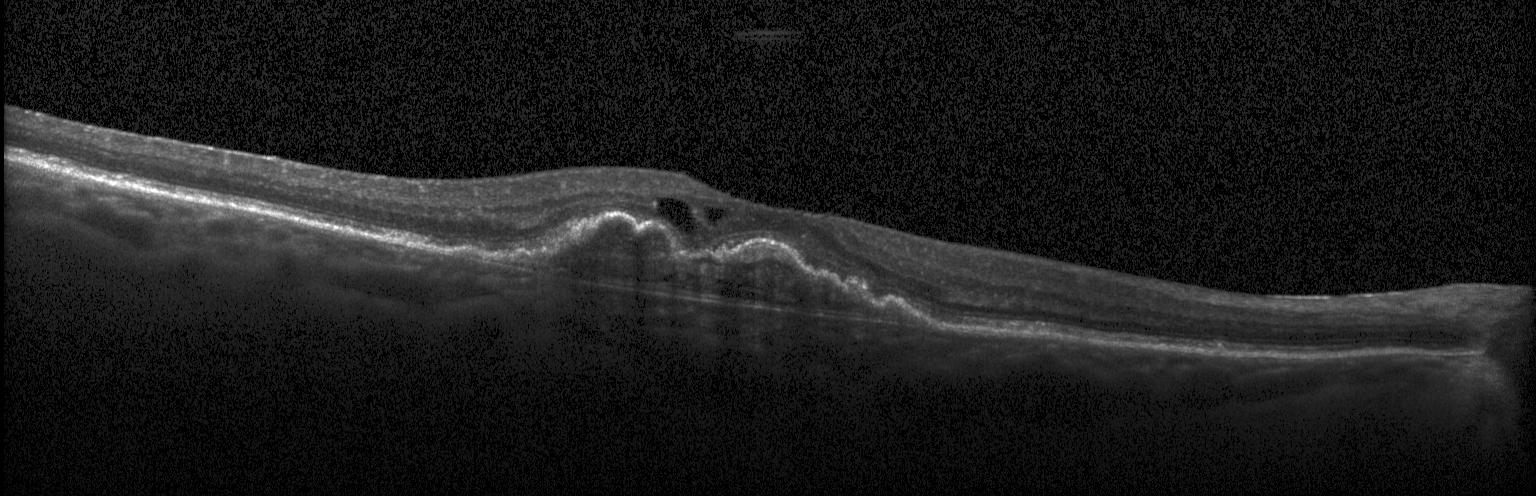

Spectral-domain optical coherence tomography; Heidelberg Spectralis OCT system; optical coherence tomography B-scan. OCT finding: a choroidal neovascular membrane.